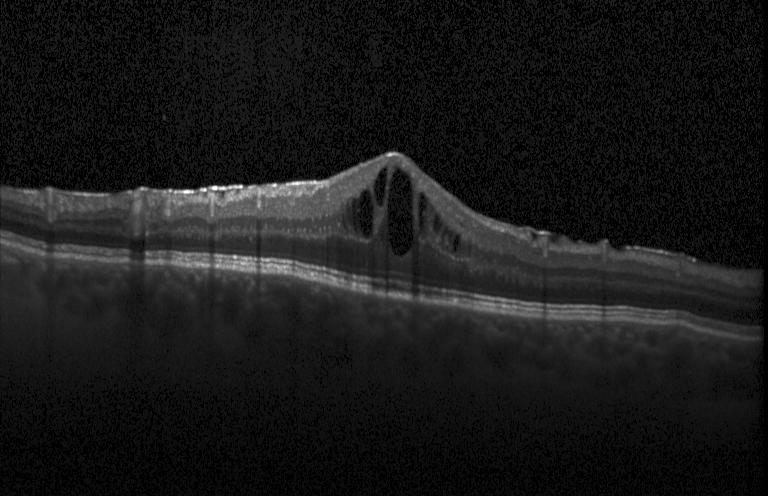
Spectral-domain OCT B-scan: DME.